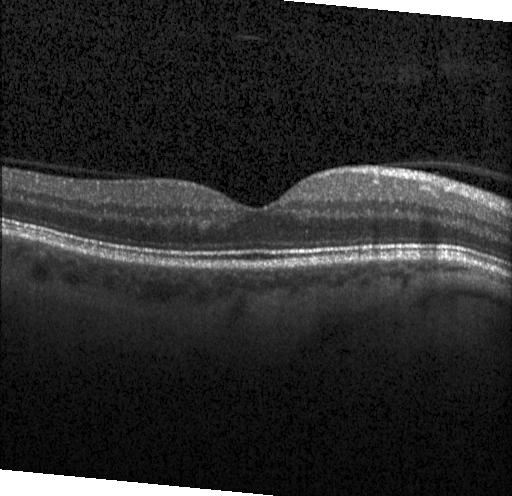 OCT scan showing neither CNV, DME, nor drusen.